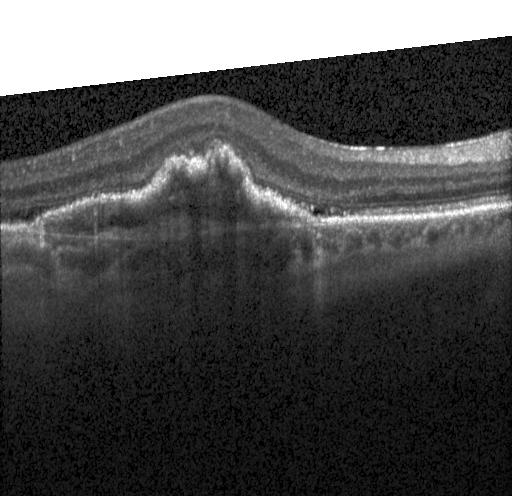 Dx: a choroidal neovascular membrane.